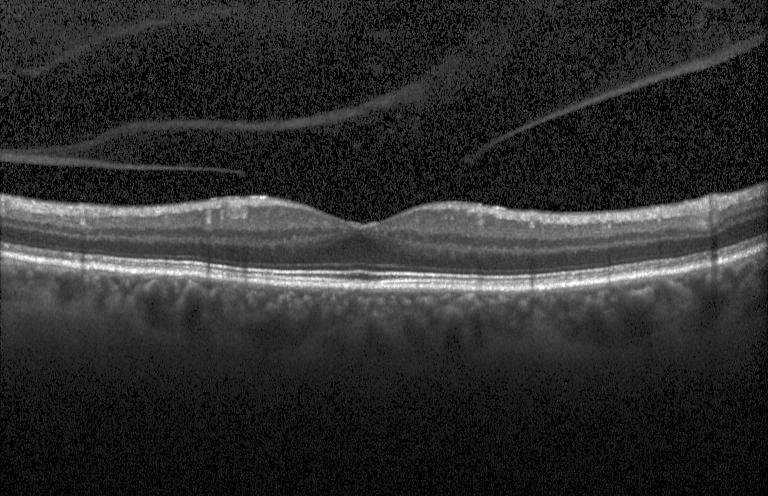
Finding: neither choroidal neovascularization, diabetic macular edema, nor drusen.